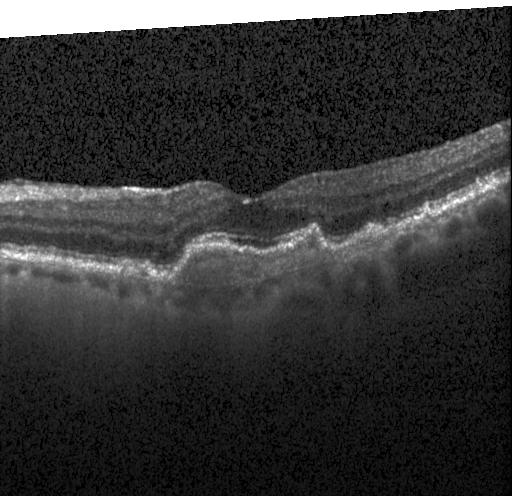

This B-scan demonstrates choroidal neovascularization (CNV).